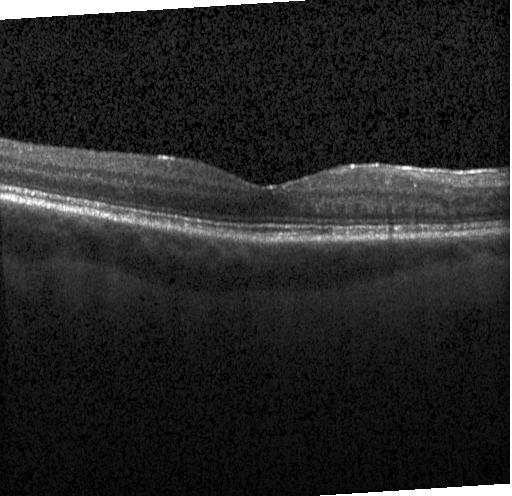

OCT B-scan showing neither choroidal neovascularization, diabetic macular edema, nor drusen.